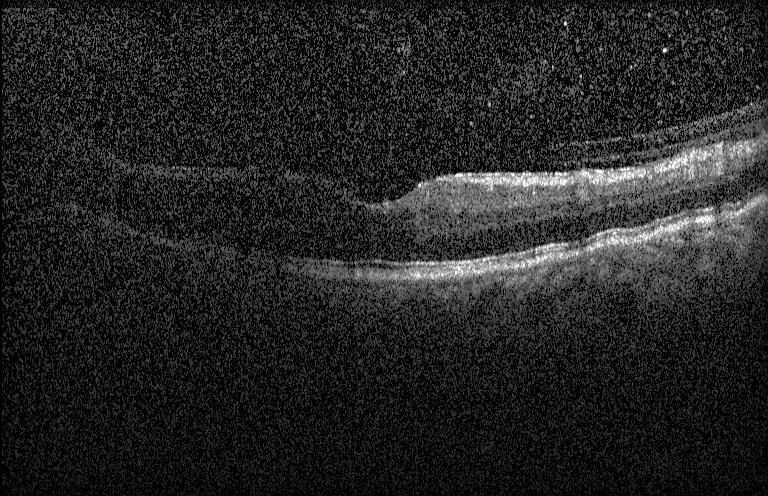 OCT line scan — This B-scan demonstrates no evidence of choroidal neovascularization, diabetic macular edema, or drusen.